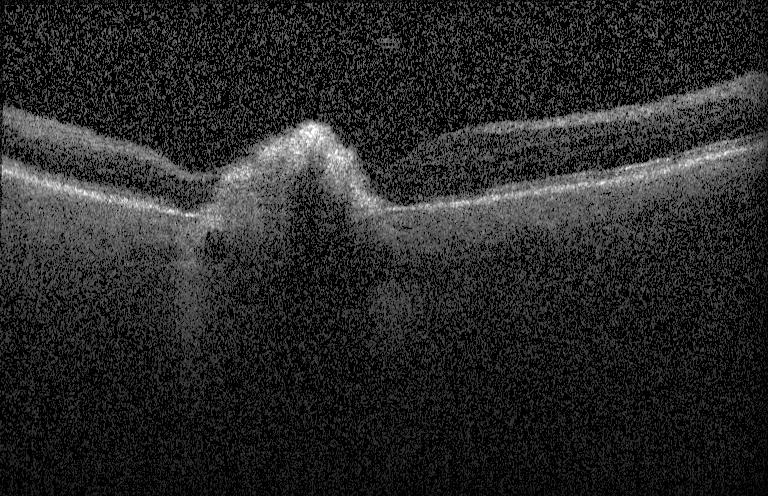

Impression: choroidal neovascularization (CNV).